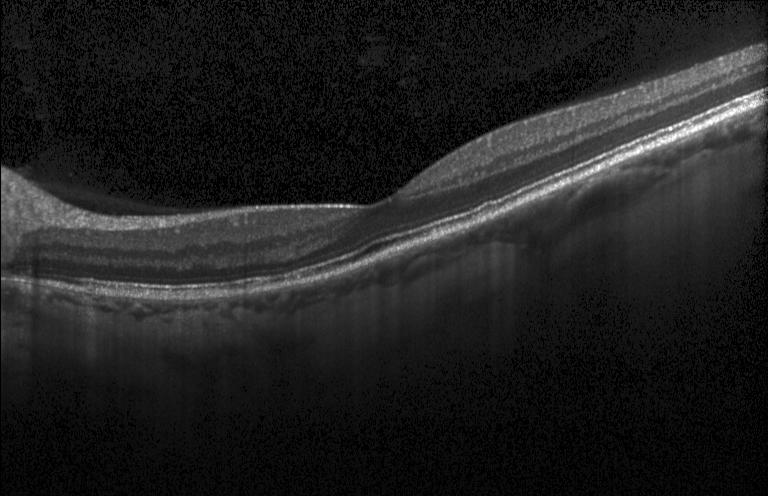

Impression: no CNV, DME, or drusen.